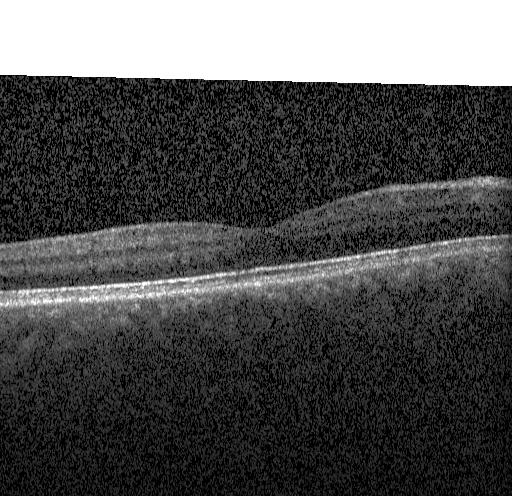 Heidelberg Spectralis · optical coherence tomography B-scan
Assessment: no choroidal neovascularization, diabetic macular edema, or drusen.